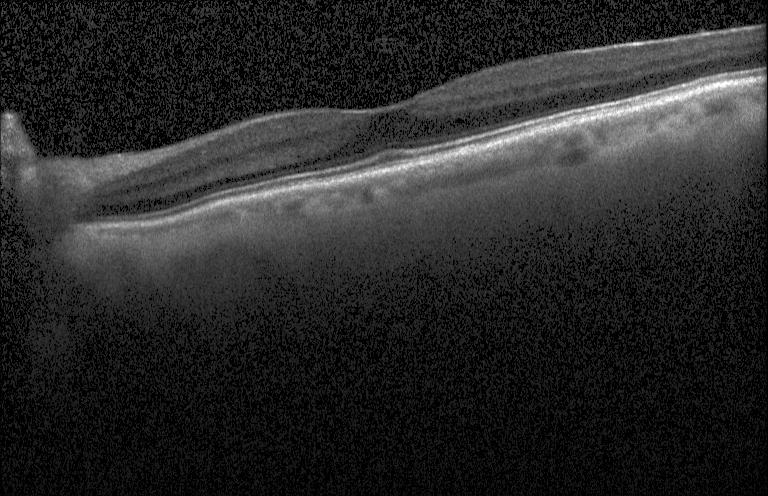

Finding: no choroidal neovascularization, no diabetic macular edema, and no drusen.